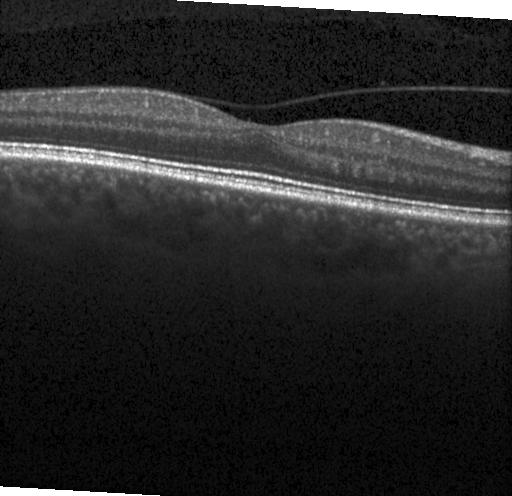

OCT line scan · SD-OCT · horizontal scan through the fovea · Heidelberg Spectralis OCT system
Macular OCT: no choroidal neovascularization, diabetic macular edema, or drusen.